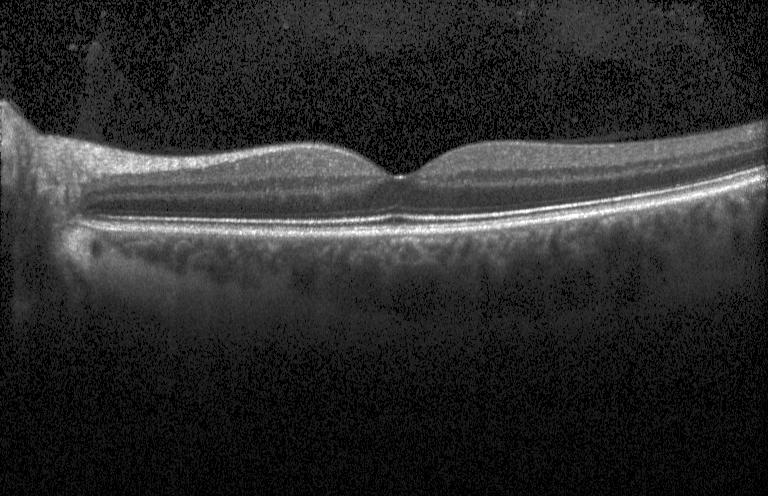
Retinal OCT cross-section showing no CNV, DME, or drusen.